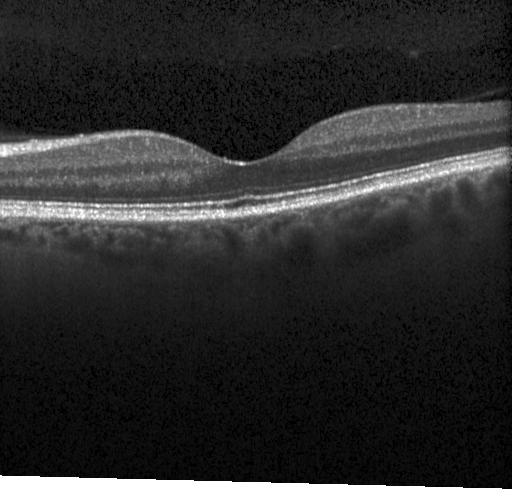
Retinal OCT cross-section showing no choroidal neovascularization, diabetic macular edema, or drusen.